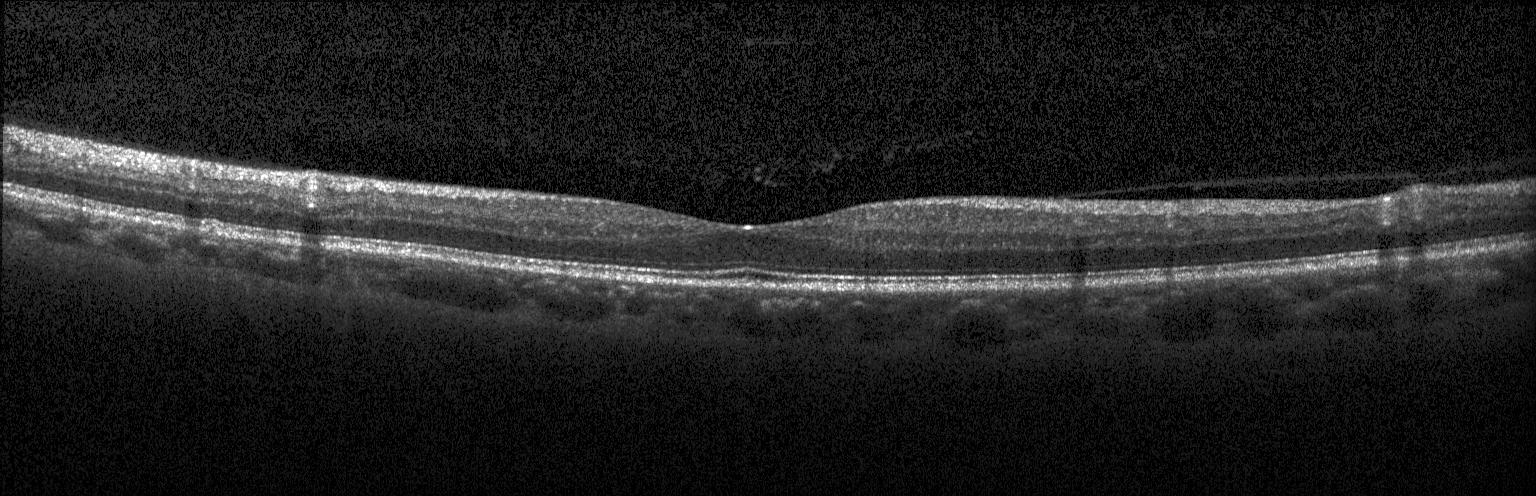

Acquired on a Heidelberg Spectralis. OCT B-scan
Finding: no evidence of choroidal neovascularization, diabetic macular edema, or drusen.